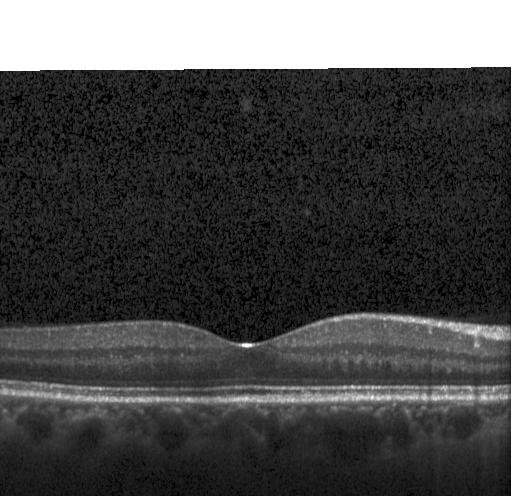 Retinal OCT cross-section — Diagnosis: no evidence of CNV, DME, or drusen.